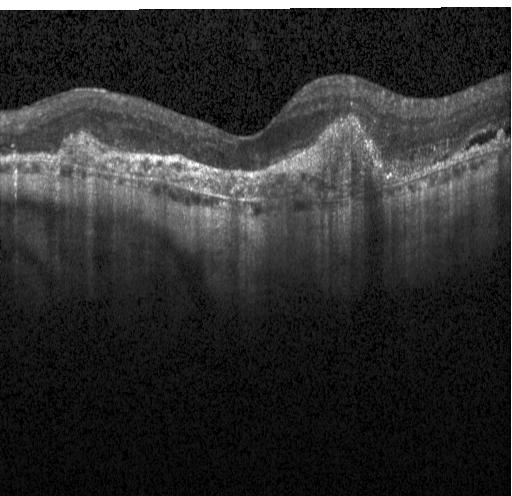

Optical coherence tomography scan, fovea-centered
This B-scan demonstrates a choroidal neovascular membrane.